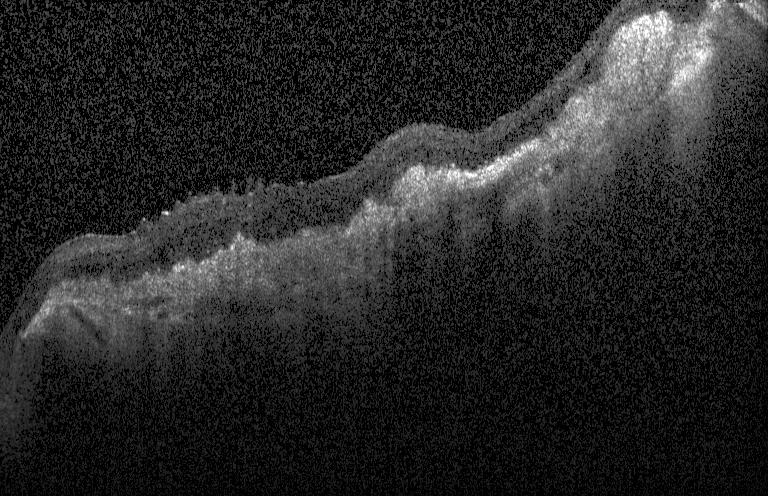 SD-OCT · OCT B-scan.
Assessment: a choroidal neovascular membrane.